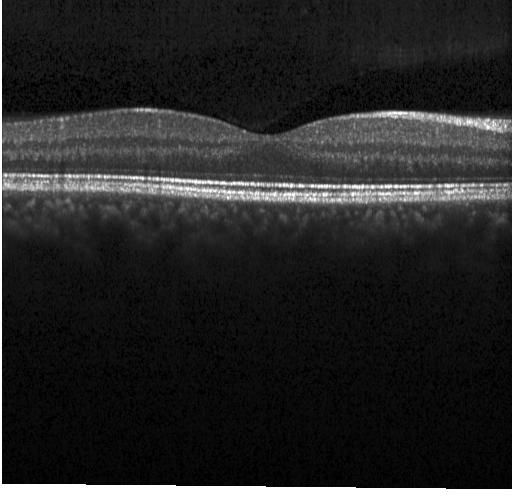 Retinal OCT cross-section showing neither choroidal neovascularization, diabetic macular edema, nor drusen.